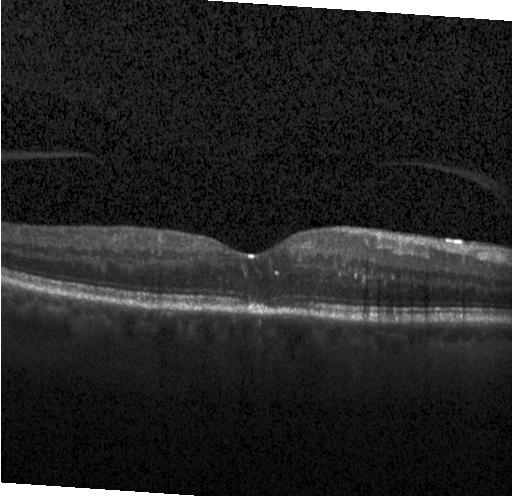
Impression: neither choroidal neovascularization, diabetic macular edema, nor drusen.